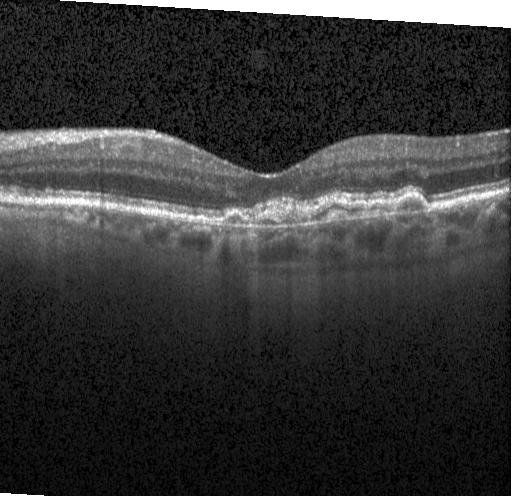

A choroidal neovascular membrane.